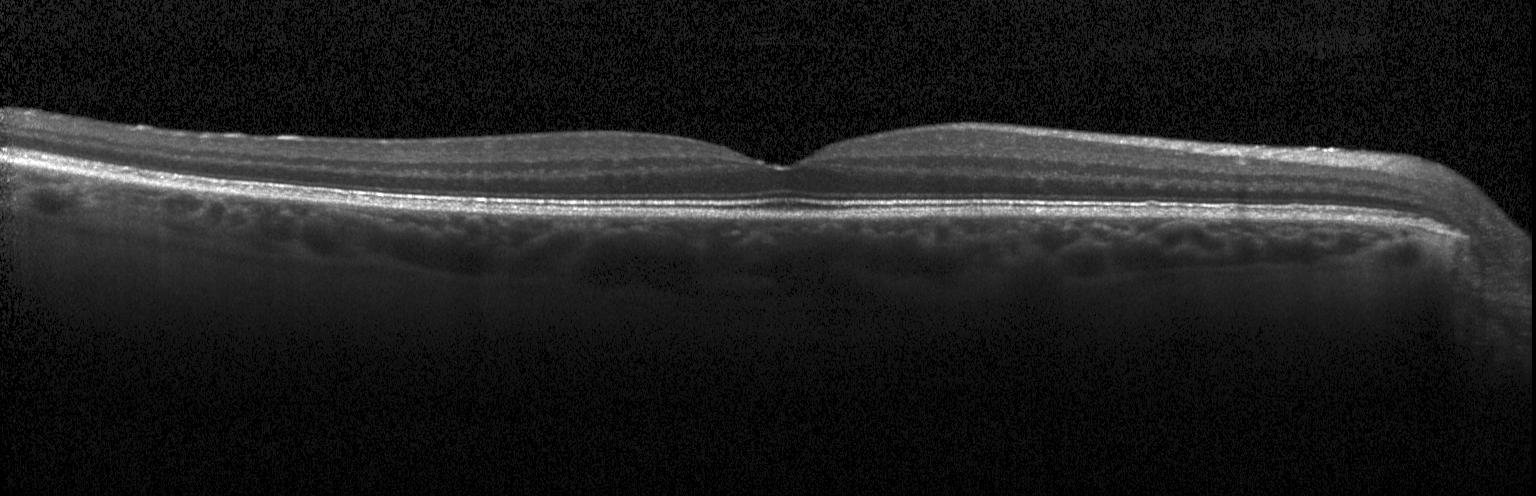

Spectral-domain OCT; horizontal scan through the fovea; retinal OCT B-scan; Heidelberg Spectralis OCT system. Impression: neither choroidal neovascularization, diabetic macular edema, nor drusen.